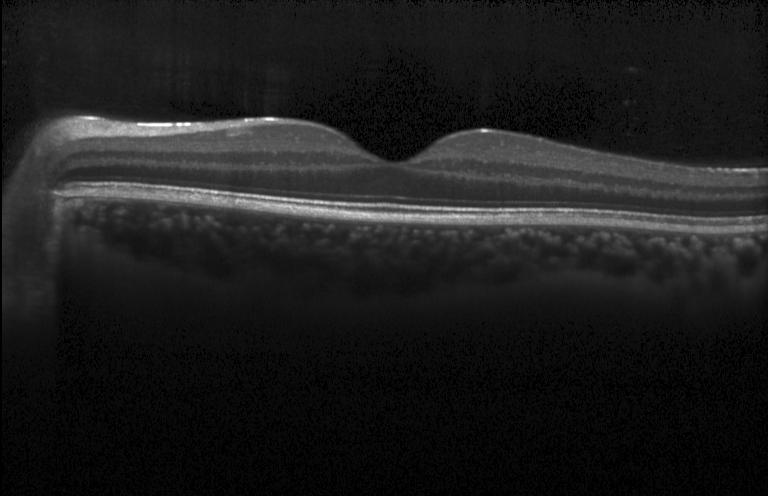

The scan shows neither choroidal neovascularization, diabetic macular edema, nor drusen.